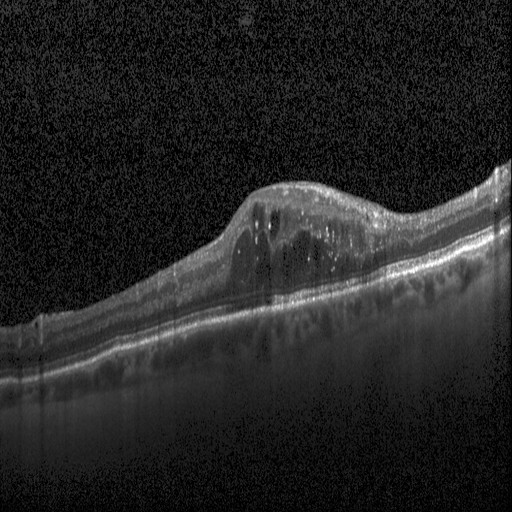 DME.